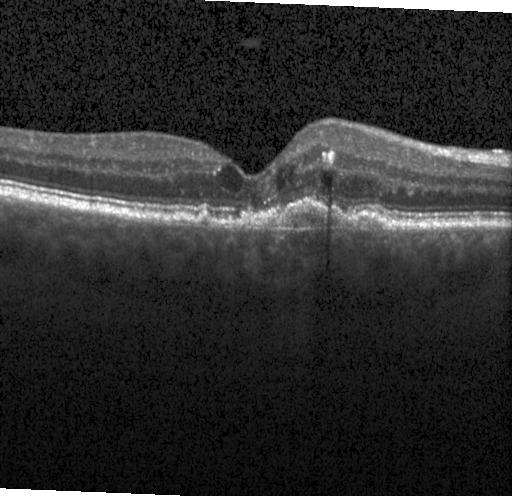 Macular OCT demonstrating a choroidal neovascular membrane.